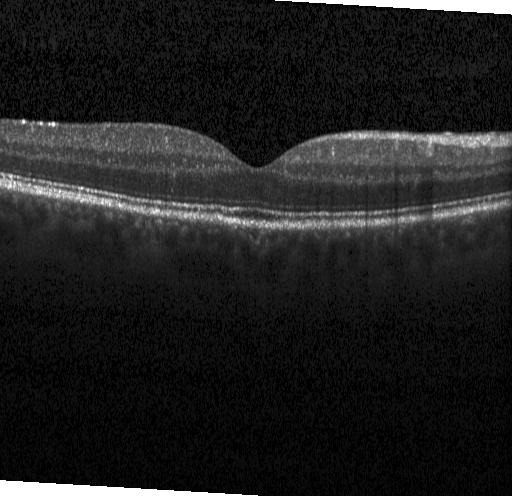 Centered on the fovea, OCT line scan.
This B-scan demonstrates no CNV, DME, or drusen.